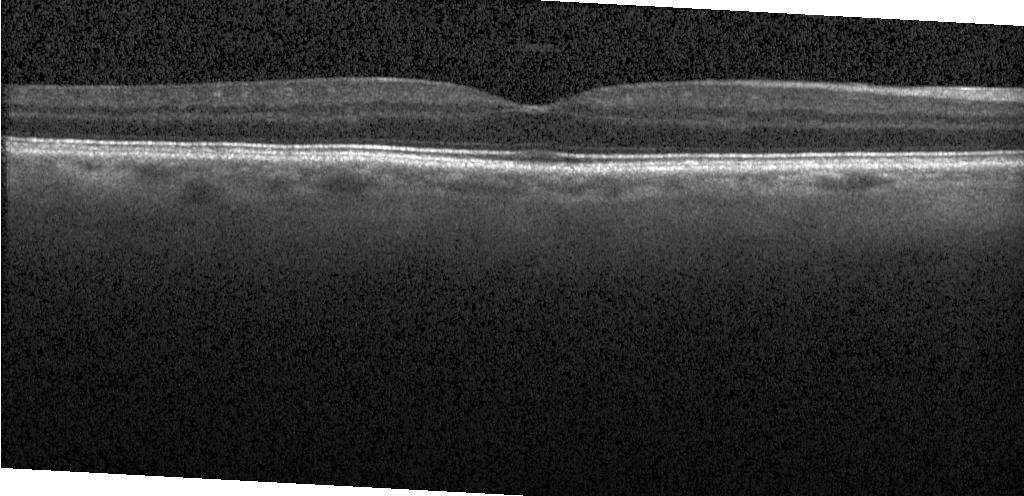
Retinal OCT B-scan; spectral-domain optical coherence tomography.
The scan shows no evidence of choroidal neovascularization, diabetic macular edema, or drusen.